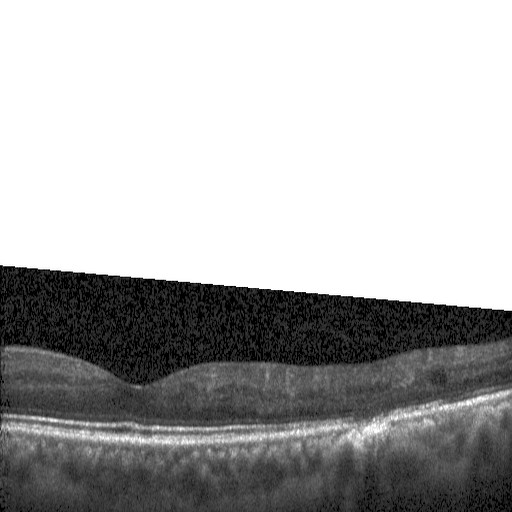

Macular OCT: DME.